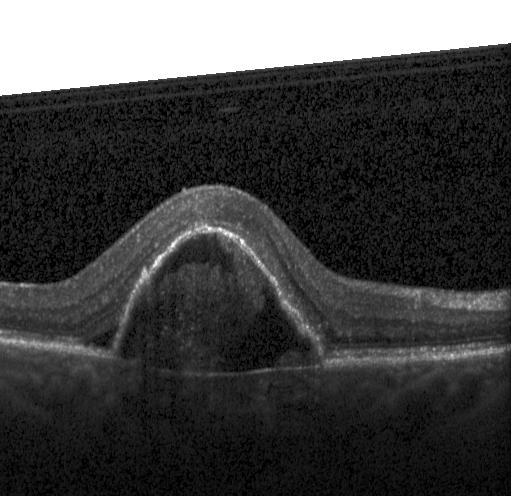 Spectral-domain OCT B-scan: choroidal neovascularization.